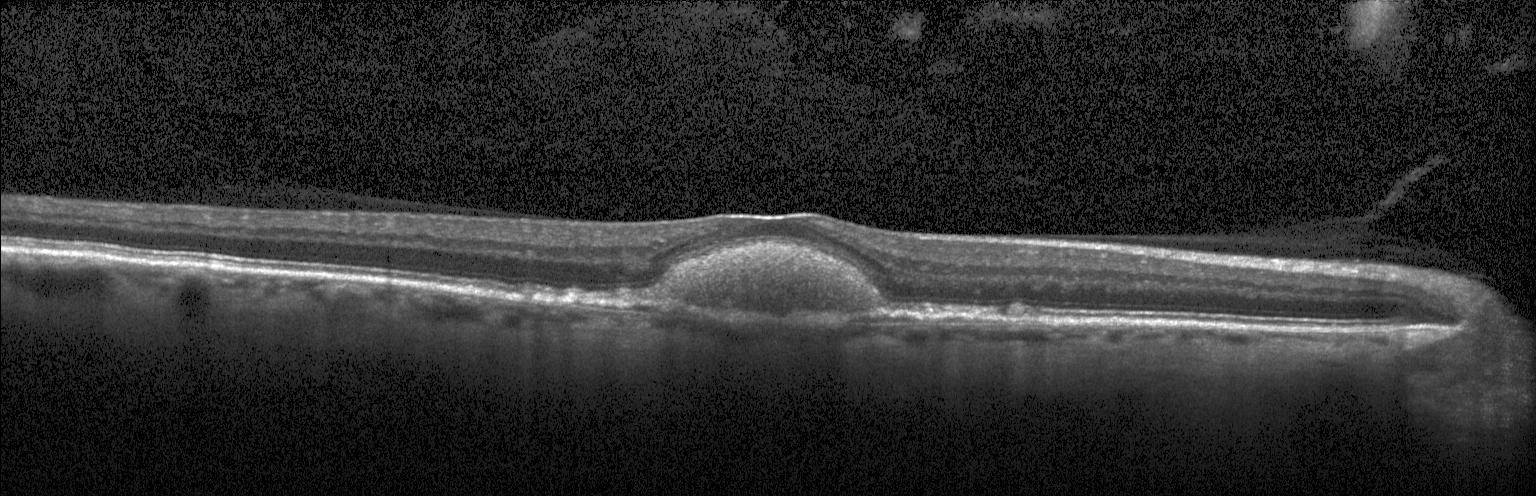 Retinal OCT cross-section showing CNV.